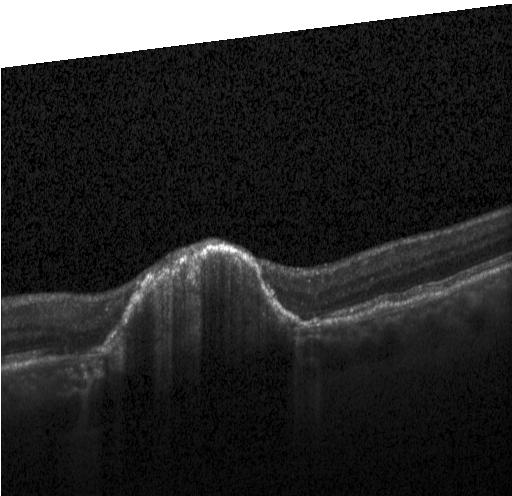 Heidelberg Spectralis · OCT B-scan. Diagnosis: CNV.